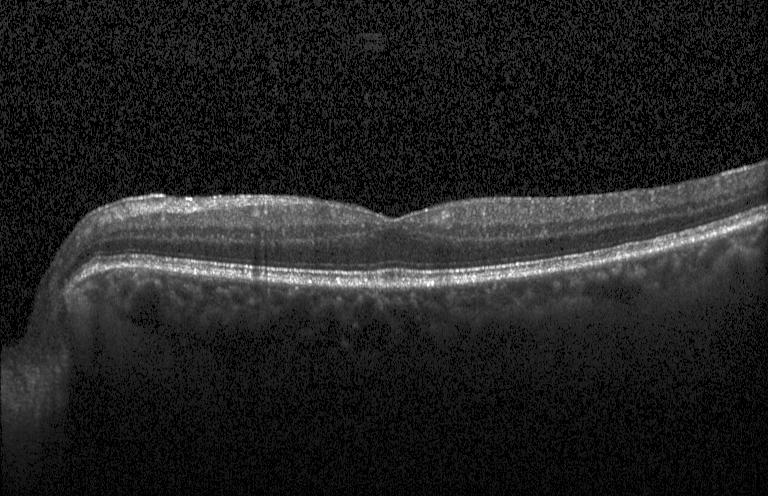 Optical coherence tomography scan
This B-scan demonstrates neither choroidal neovascularization, diabetic macular edema, nor drusen.